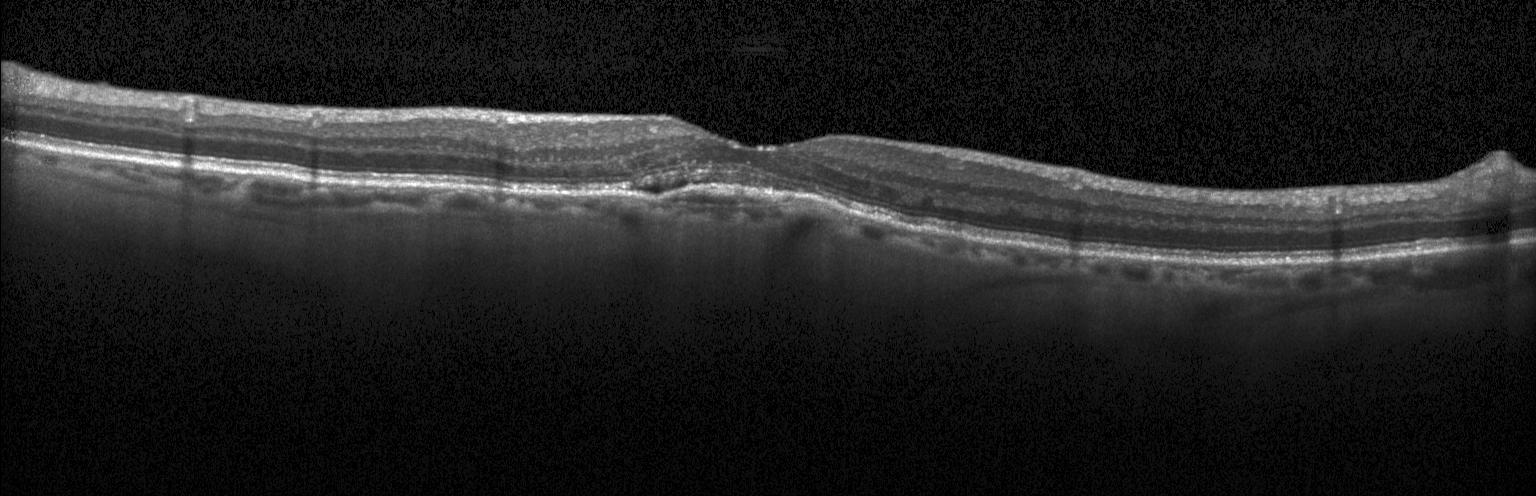 Spectral-domain OCT. Heidelberg Spectralis OCT system. Retinal OCT B-scan
Impression: a choroidal neovascular membrane.